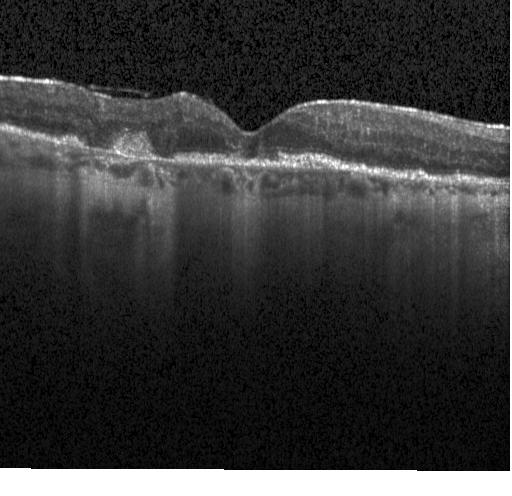

Retinal OCT B-scan — Assessment: a choroidal neovascular membrane.